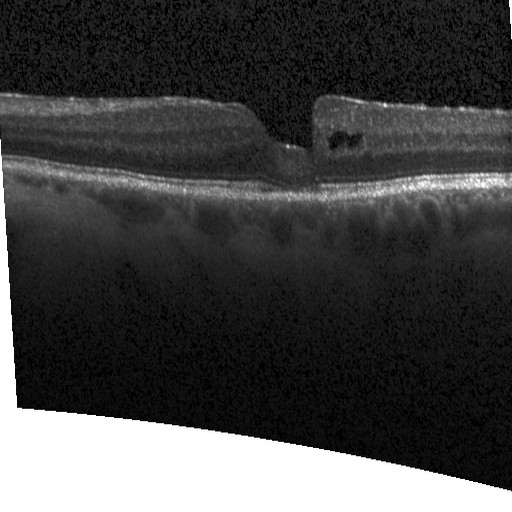

Diagnosis: diabetic macular edema.